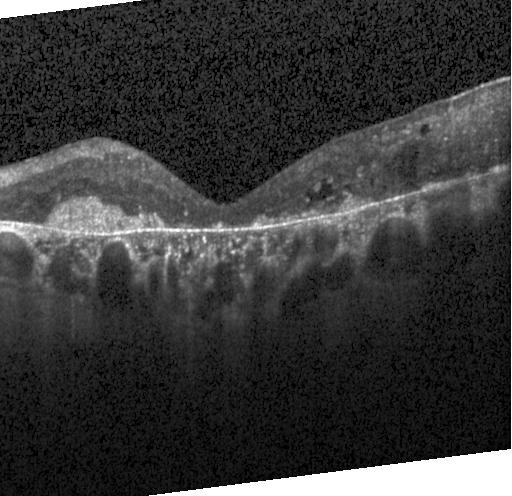
OCT scan showing a choroidal neovascular membrane.